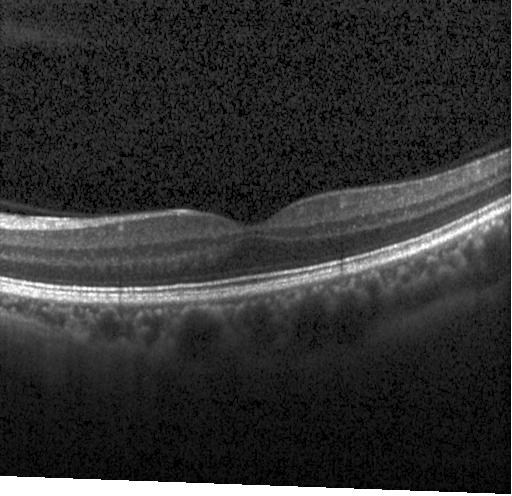
OCT B-scan; spectral-domain OCT; instrument: Heidelberg Spectralis — This B-scan demonstrates no choroidal neovascularization, no diabetic macular edema, and no drusen.